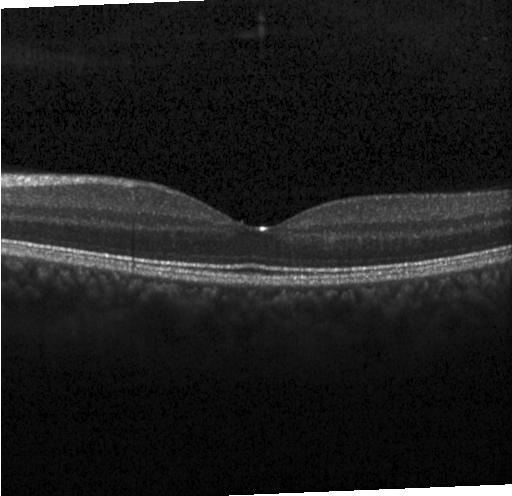

Retinal OCT cross-section showing neither choroidal neovascularization, diabetic macular edema, nor drusen.